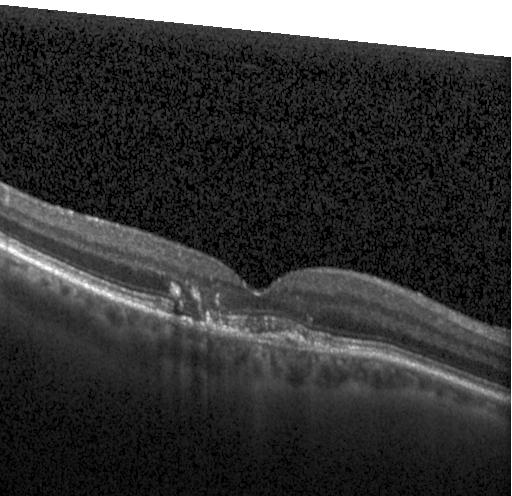 Heidelberg Spectralis · spectral-domain OCT · retinal OCT cross-section. The scan shows a choroidal neovascular membrane.